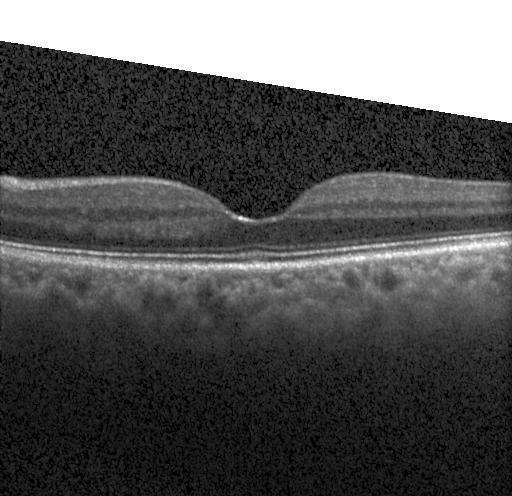 Optical coherence tomography scan.
Impression: no choroidal neovascularization, diabetic macular edema, or drusen.